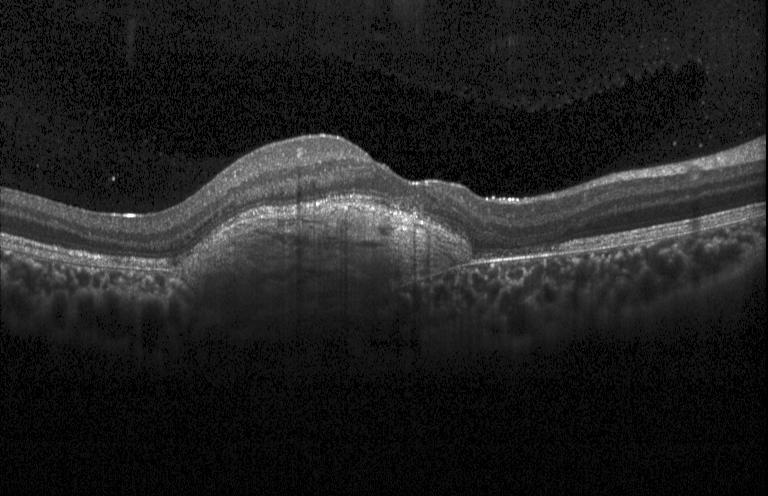
Diagnosis: a choroidal neovascular membrane.